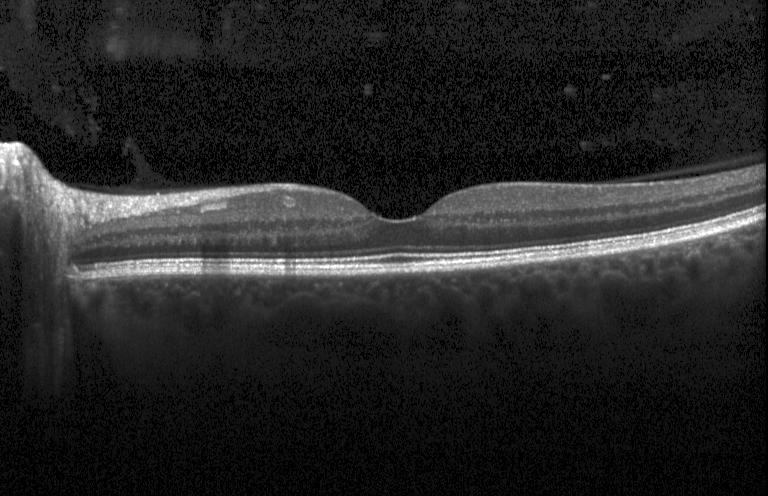
Retinal OCT cross-section · Heidelberg Spectralis · spectral-domain optical coherence tomography · through the macula
The scan shows no CNV, DME, or drusen.